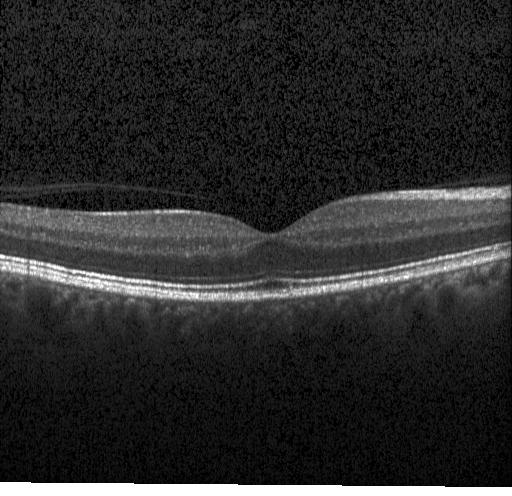

Spectral-domain OCT, Heidelberg Spectralis OCT system, retinal OCT cross-section, through the macula — Dx: no CNV, no DME, and no drusen.